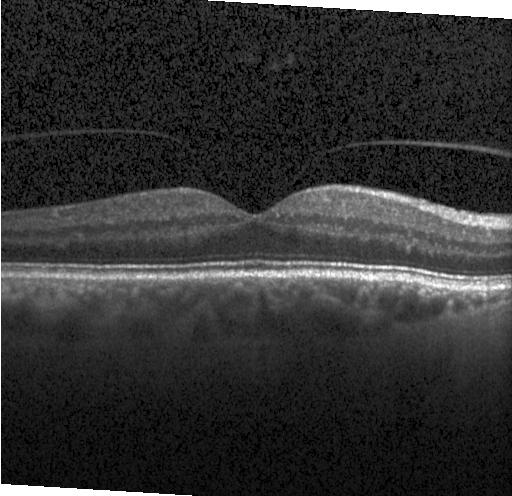 Finding: no evidence of choroidal neovascularization, diabetic macular edema, or drusen.